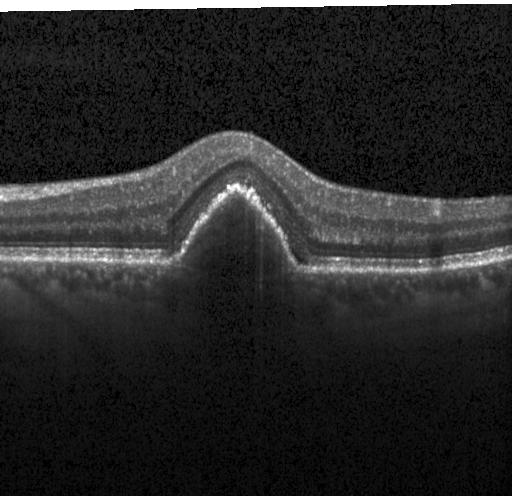
Spectral-domain OCT; Heidelberg Spectralis OCT system; retinal OCT B-scan. Macular OCT: CNV.